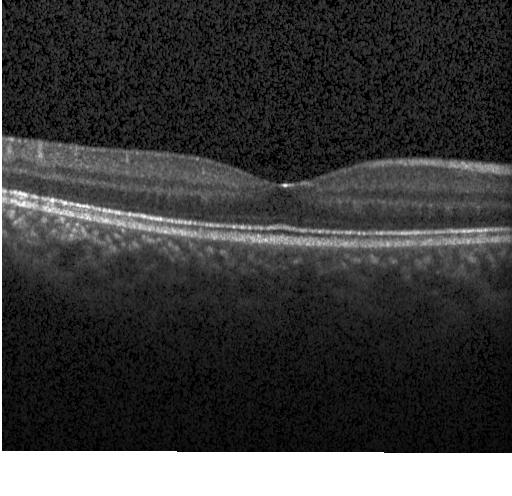

OCT B-scan showing no choroidal neovascularization, no diabetic macular edema, and no drusen.